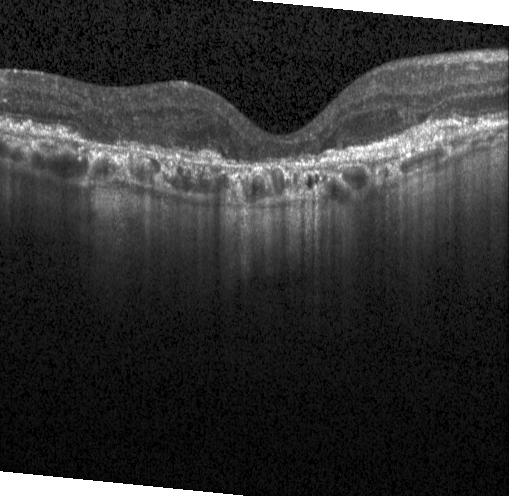
Through the macula. Spectral-domain optical coherence tomography. Retinal OCT B-scan. Heidelberg Spectralis OCT system
Impression: a choroidal neovascular membrane.